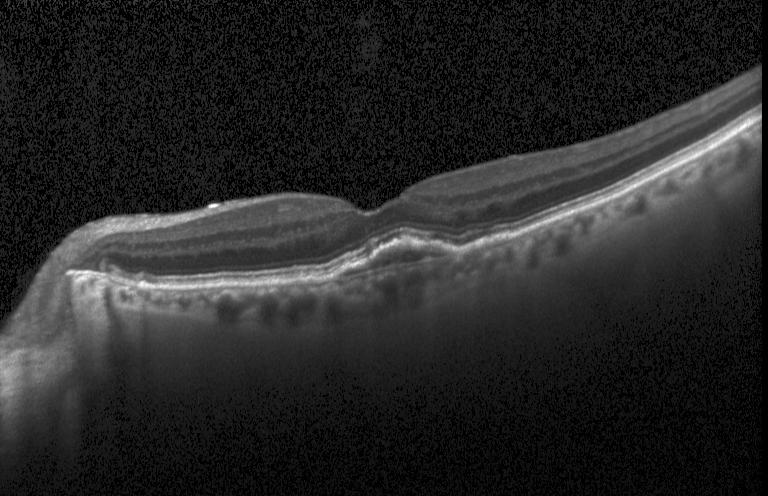

Impression: a choroidal neovascular membrane.